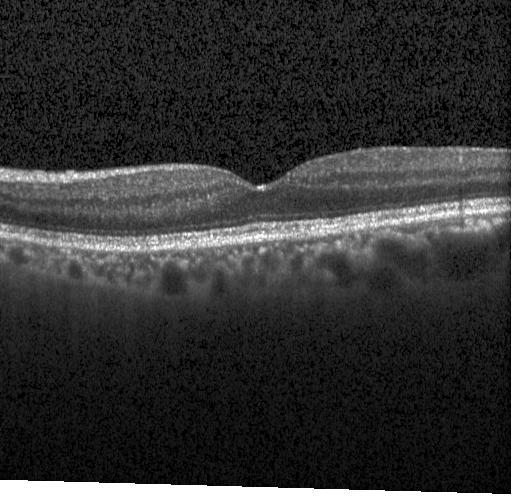 Impression: neither choroidal neovascularization, diabetic macular edema, nor drusen.